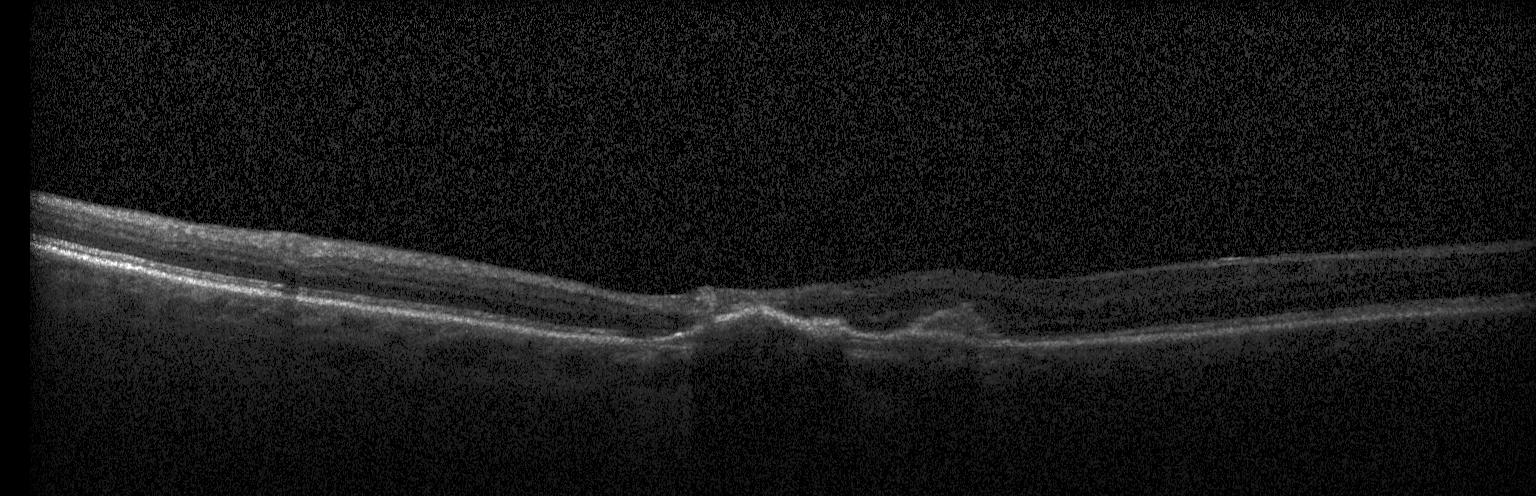

Optical coherence tomography scan.
Impression: a choroidal neovascular membrane.